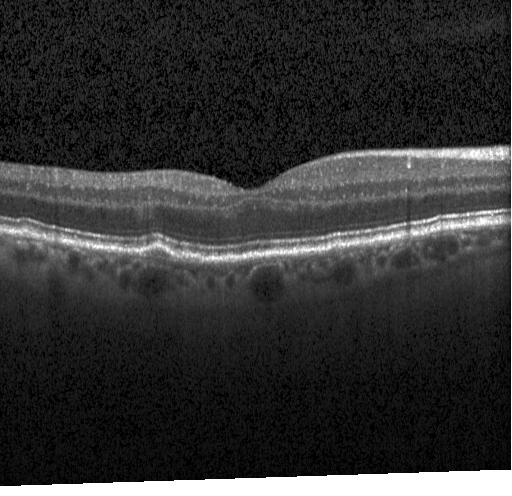

Retinal OCT B-scan.
Finding: multiple drusen.